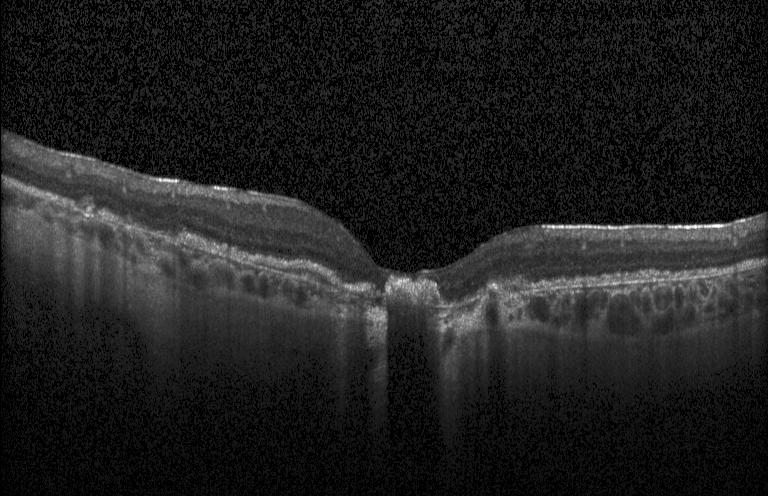

Optical coherence tomography scan. The scan shows a choroidal neovascular membrane.